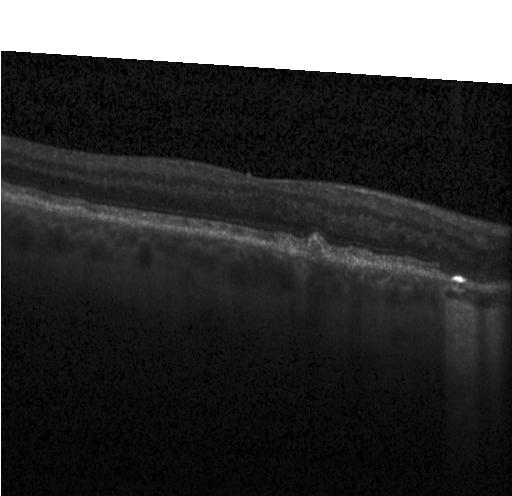
Retinal OCT B-scan. Spectral-domain optical coherence tomography. Horizontal scan through the fovea. Heidelberg Spectralis.
Finding: sub-RPE drusenoid deposits.